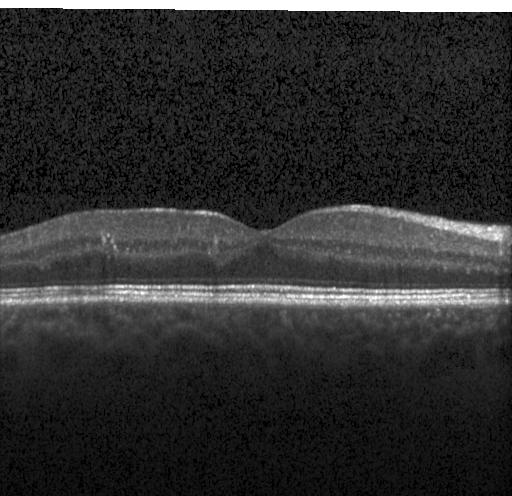
Acquired on a Heidelberg Spectralis. Optical coherence tomography B-scan.
Impression: no CNV, no DME, and no drusen.